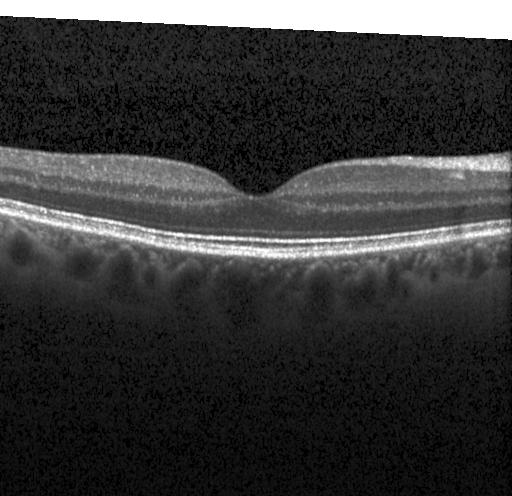 No choroidal neovascularization, no diabetic macular edema, and no drusen.